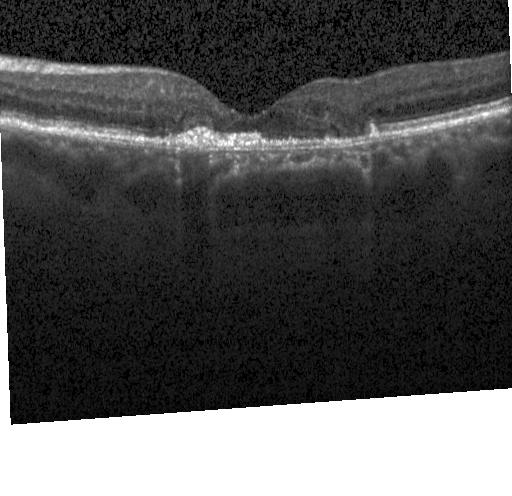
OCT finding: choroidal neovascularization (CNV).